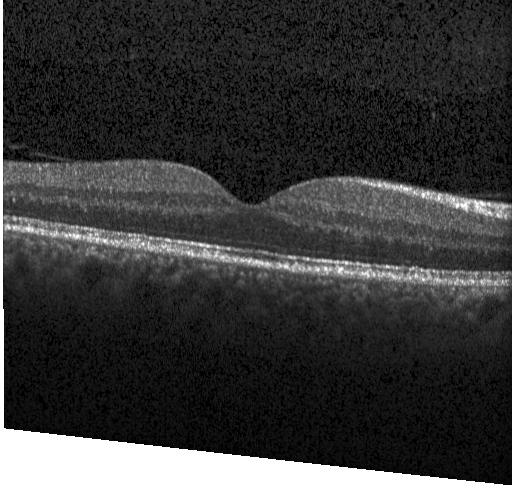
Instrument: Heidelberg Spectralis; fovea-centered; spectral-domain optical coherence tomography; retinal OCT cross-section — The scan shows no CNV, no DME, and no drusen.